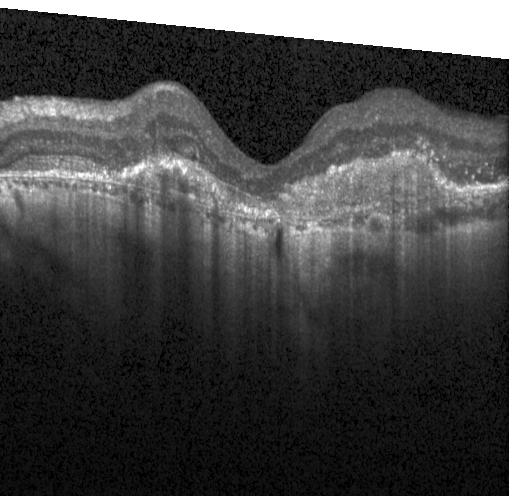

Optical coherence tomography scan · acquired on a Heidelberg Spectralis. Finding: CNV.